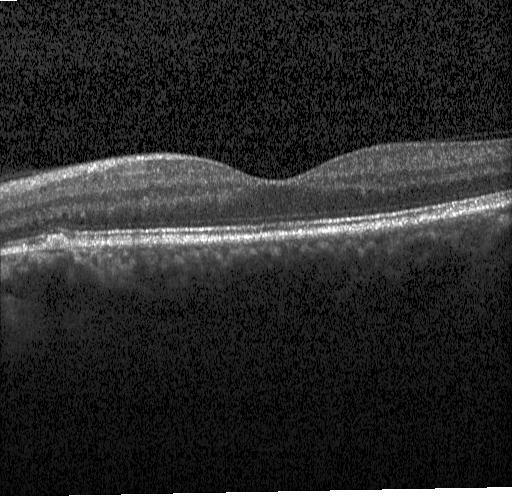

Heidelberg Spectralis OCT system. Macular scan. Spectral-domain optical coherence tomography. Retinal OCT B-scan. Finding: multiple drusen.